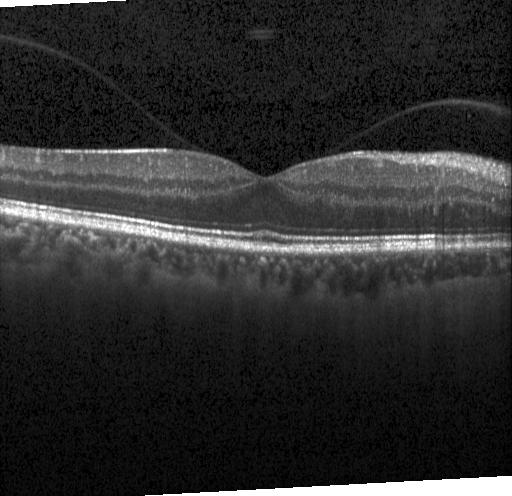
Retinal OCT cross-section; spectral-domain optical coherence tomography
Dx: no CNV, no DME, and no drusen.